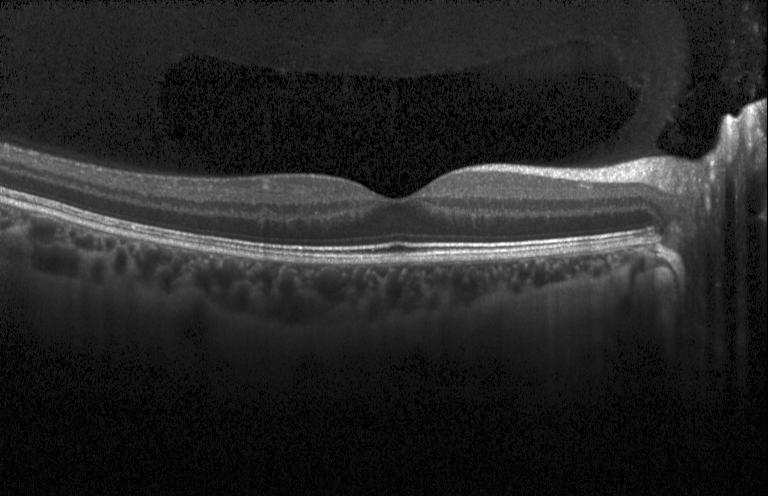

Finding: no CNV, no DME, and no drusen.